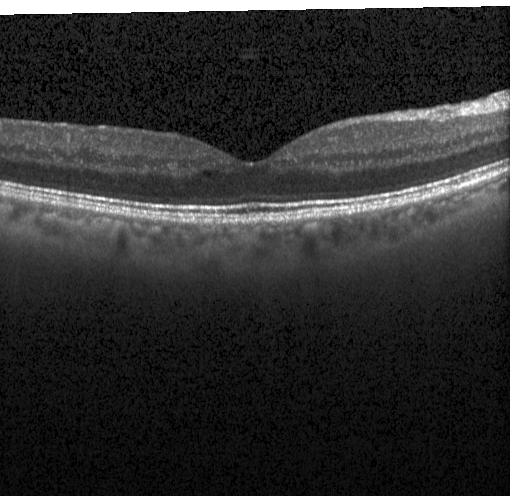
Assessment: no choroidal neovascularization, diabetic macular edema, or drusen.